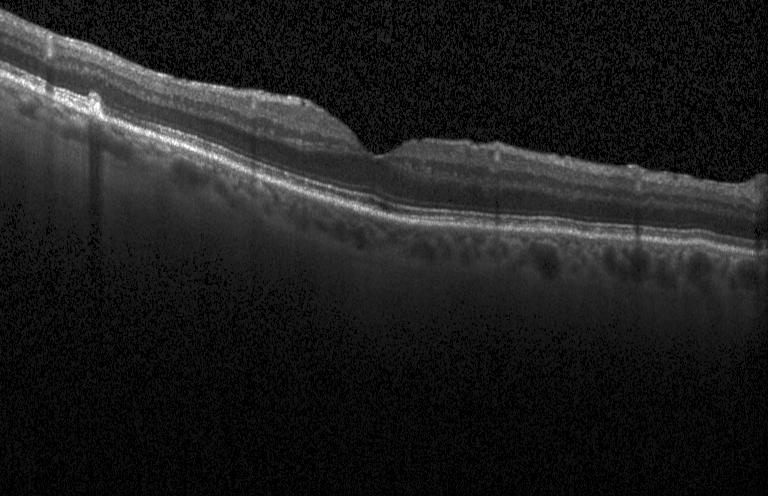

Assessment: sub-RPE drusenoid deposits.